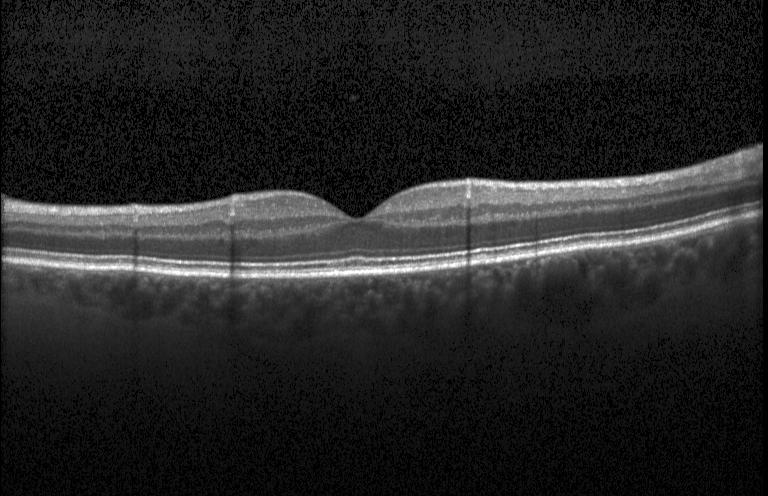
Optical coherence tomography scan, spectral-domain OCT — Assessment: no choroidal neovascularization, no diabetic macular edema, and no drusen.